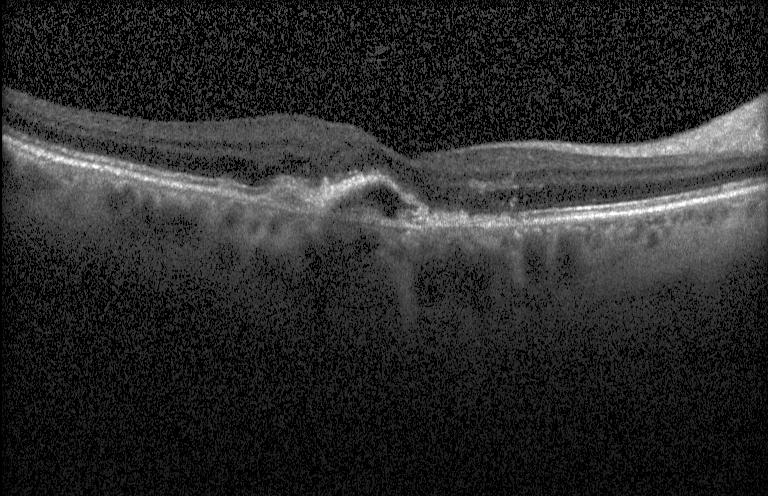

Macular OCT: a choroidal neovascular membrane.